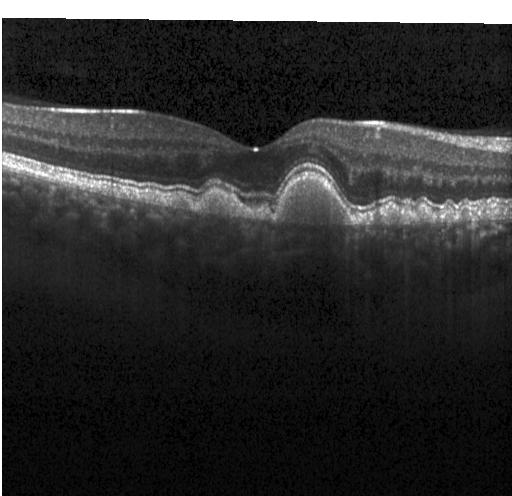
Optical coherence tomography B-scan, SD-OCT — Finding: multiple drusen.